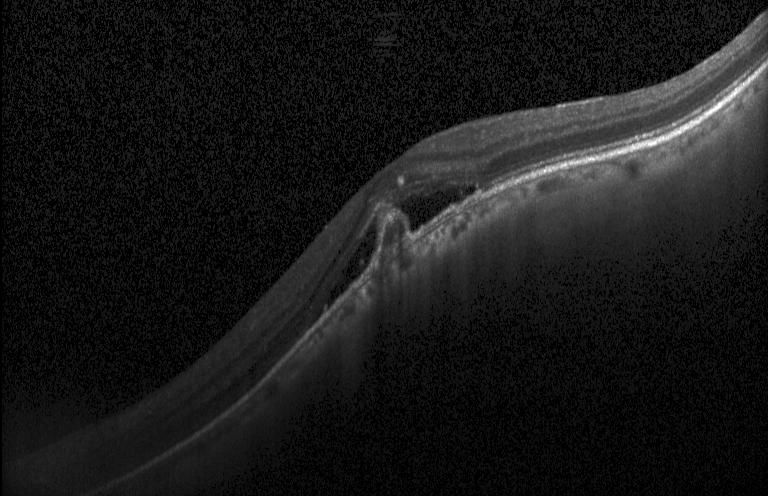

Retinal OCT B-scan.
Diagnosis: a choroidal neovascular membrane.